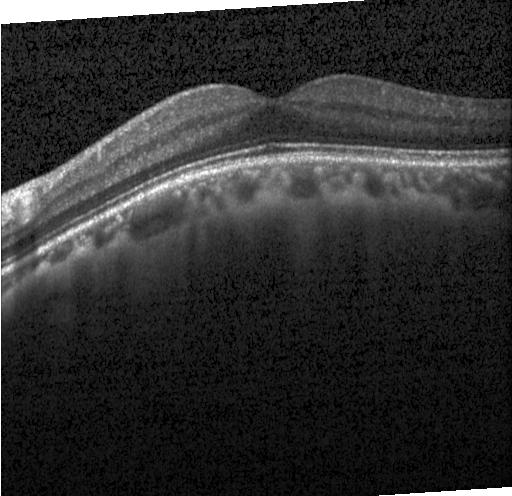

Finding: neither choroidal neovascularization, diabetic macular edema, nor drusen.